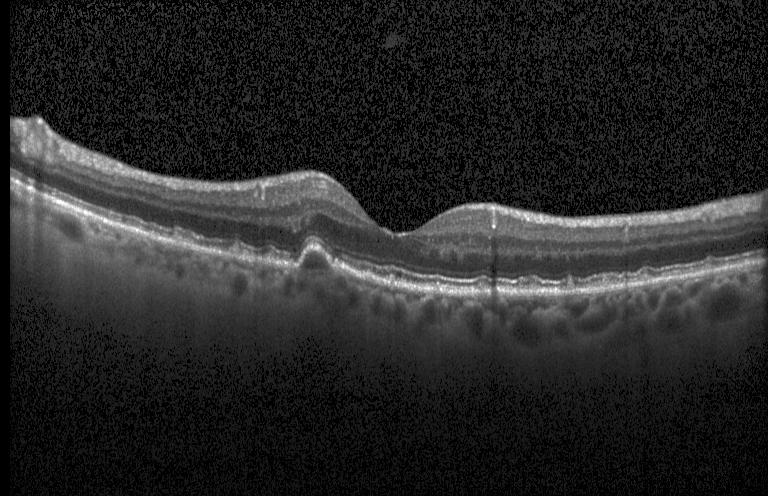 Impression: multiple drusen.